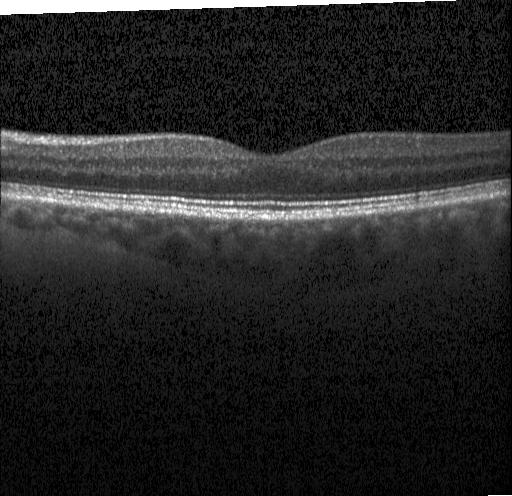

OCT line scan; spectral-domain OCT.
OCT finding: neither choroidal neovascularization, diabetic macular edema, nor drusen.